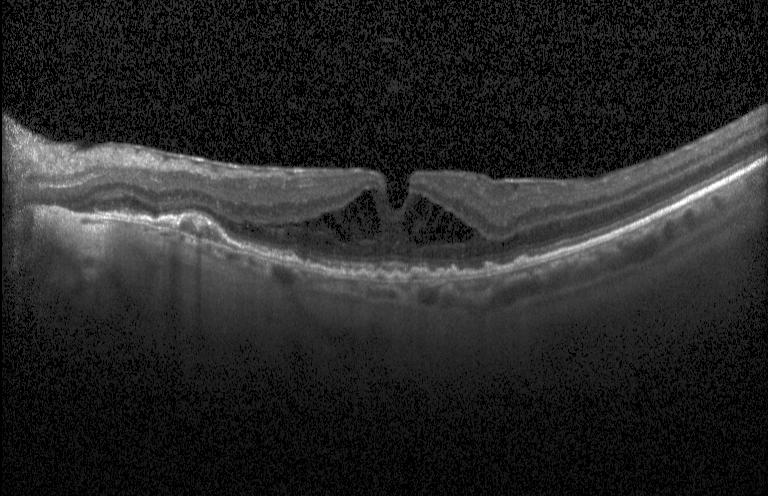
Retinal OCT B-scan · spectral-domain optical coherence tomography · horizontal scan through the fovea — Finding: DME.